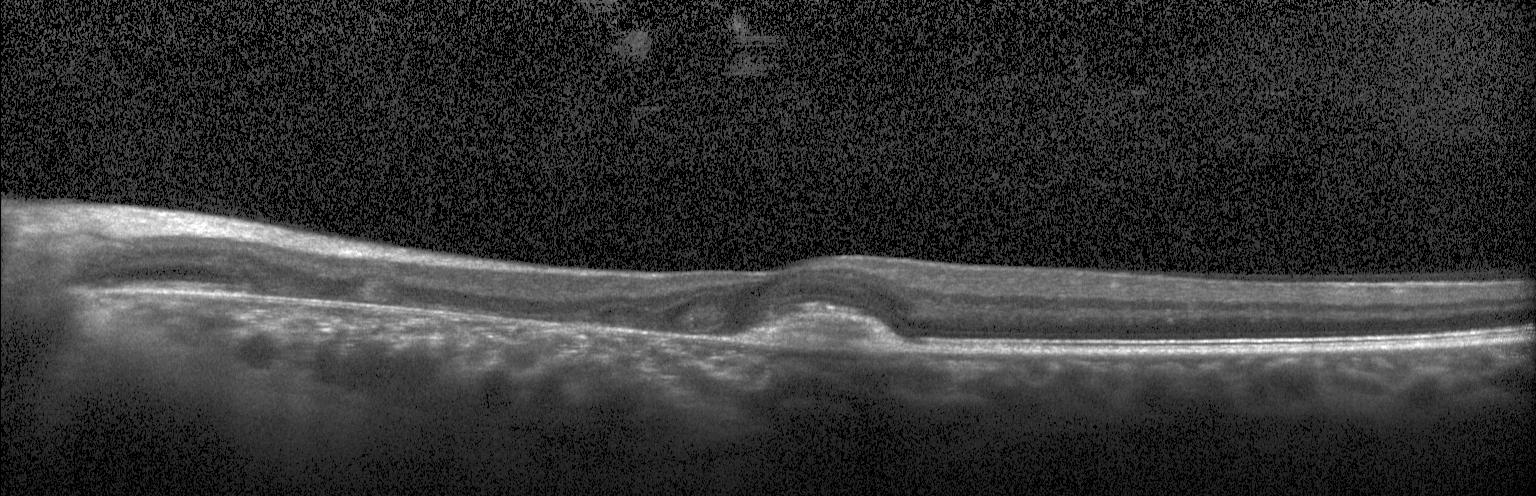 OCT scan showing a choroidal neovascular membrane.